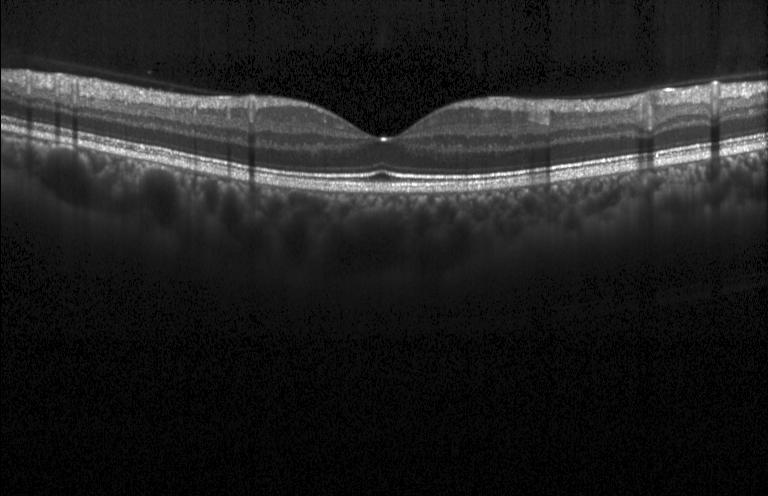
Finding: no evidence of CNV, DME, or drusen.